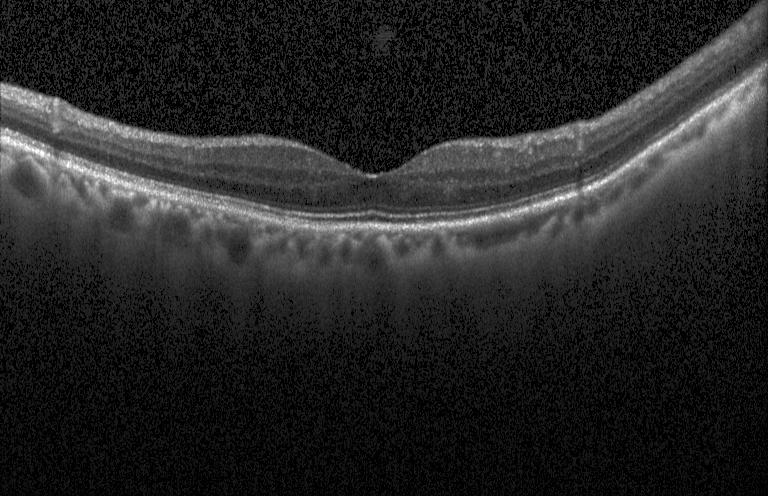

Fovea-centered; Heidelberg Spectralis OCT system; SD-OCT; retinal OCT cross-section. Impression: neither choroidal neovascularization, diabetic macular edema, nor drusen.